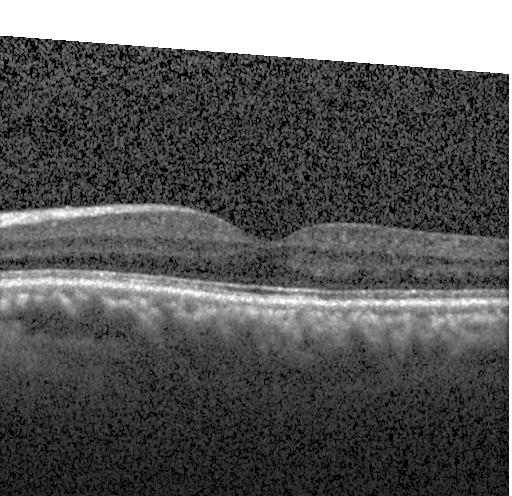 Macular OCT: neither choroidal neovascularization, diabetic macular edema, nor drusen.